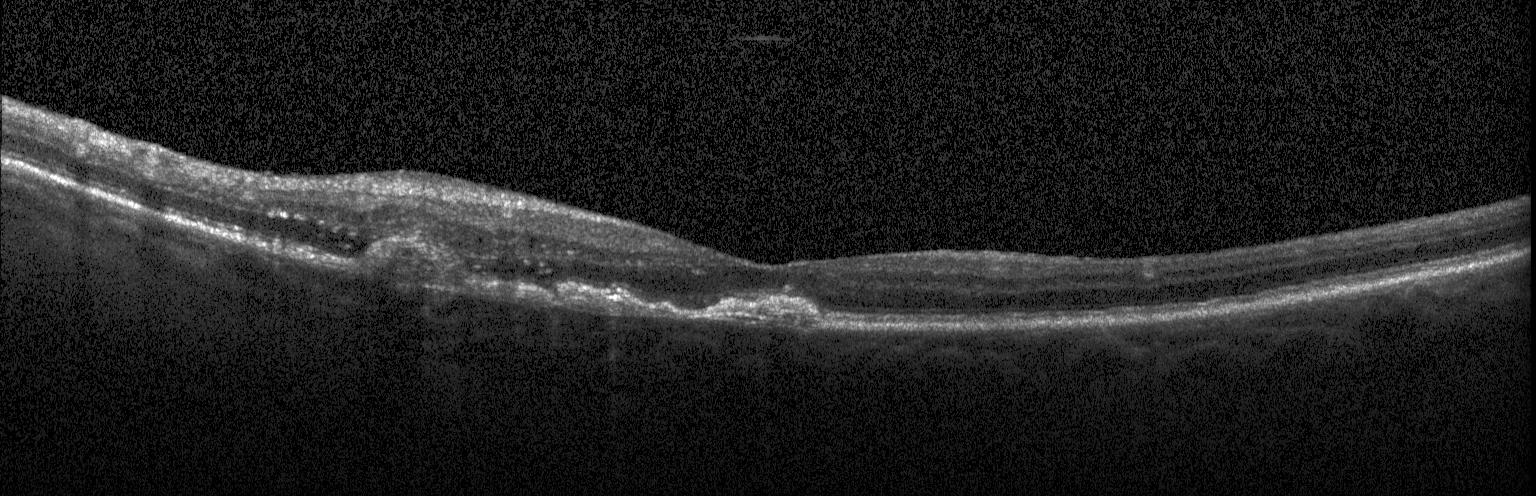
OCT B-scan, acquired on a Heidelberg Spectralis, SD-OCT
Assessment: choroidal neovascularization (CNV).